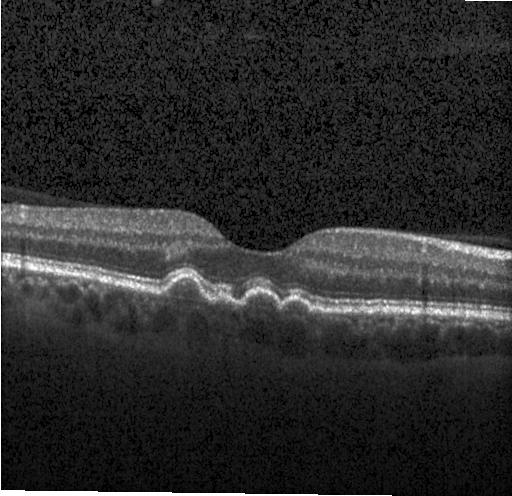 Heidelberg Spectralis · optical coherence tomography B-scan · macular scan — Macular OCT: drusen.